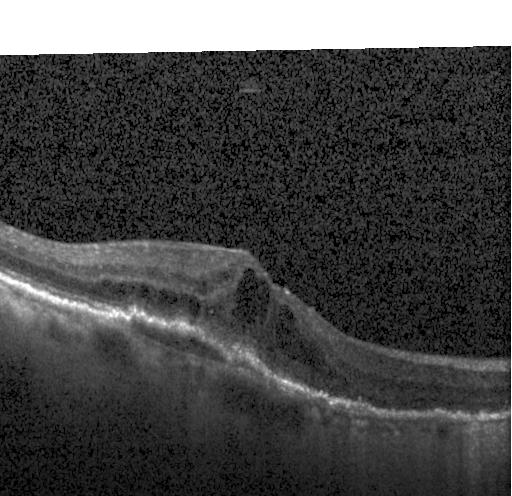

Fovea-centered; retinal OCT cross-section; acquired on a Heidelberg Spectralis.
The scan shows a choroidal neovascular membrane.